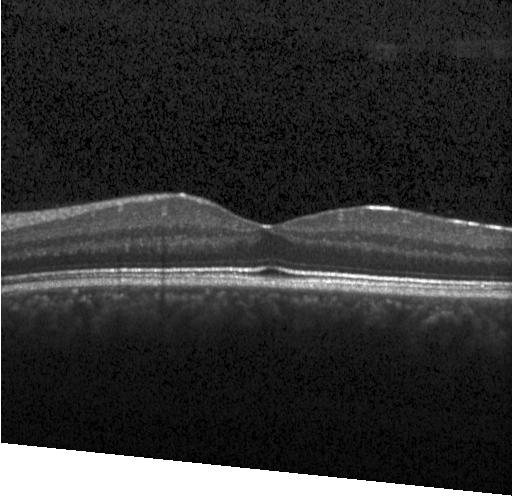

Acquired on a Heidelberg Spectralis · retinal OCT B-scan — The scan shows neither choroidal neovascularization, diabetic macular edema, nor drusen.